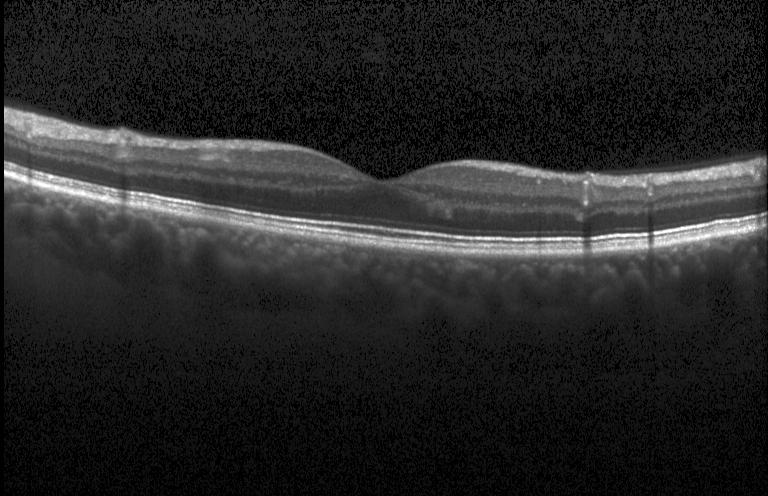 Macular OCT demonstrating no choroidal neovascularization, diabetic macular edema, or drusen.